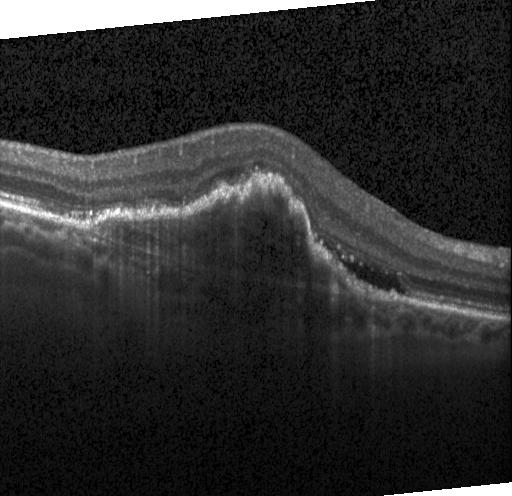 Heidelberg Spectralis. Spectral-domain OCT. OCT B-scan. Macular scan — The scan shows a choroidal neovascular membrane.